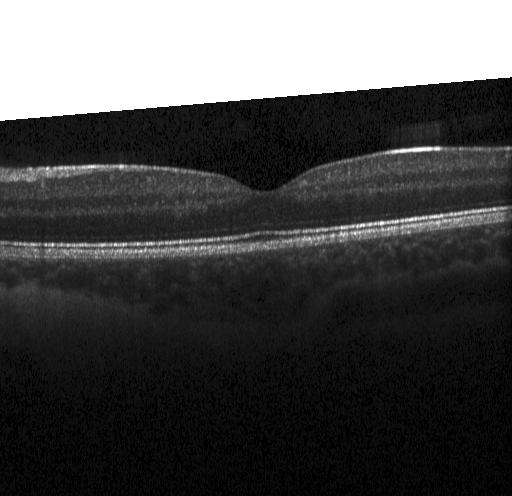 Optical coherence tomography B-scan. Through the macula — Diagnosis: no CNV, DME, or drusen.